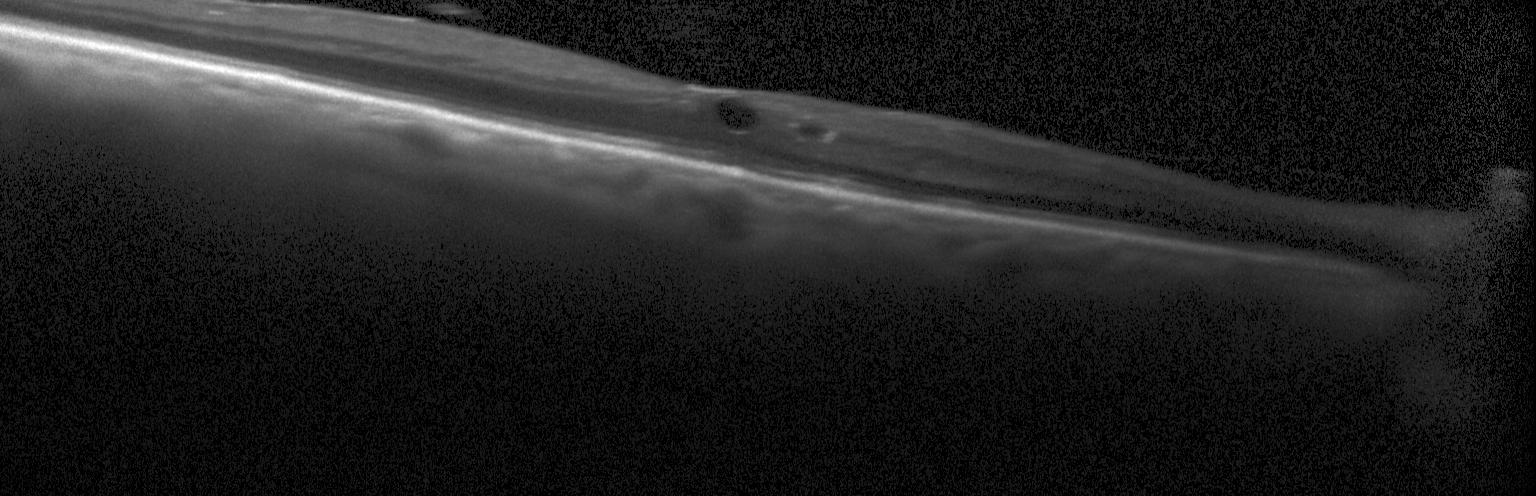

This B-scan demonstrates diabetic macular edema.